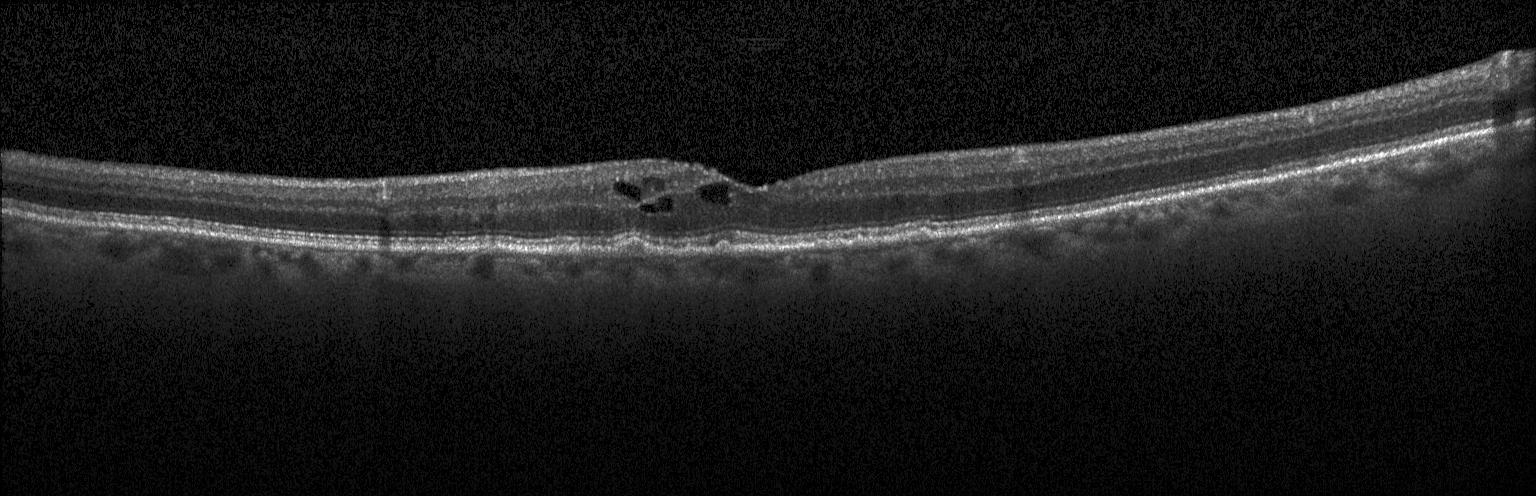 Macular OCT demonstrating diabetic macular edema.